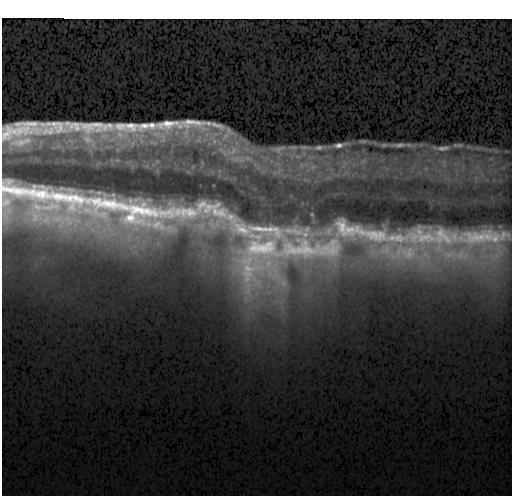 Assessment: a choroidal neovascular membrane.